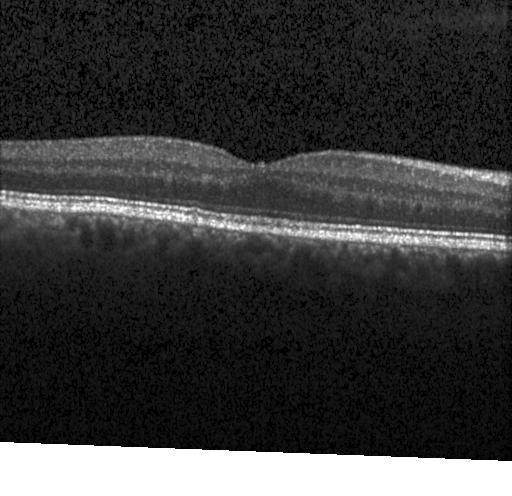
OCT scan showing no choroidal neovascularization, diabetic macular edema, or drusen.